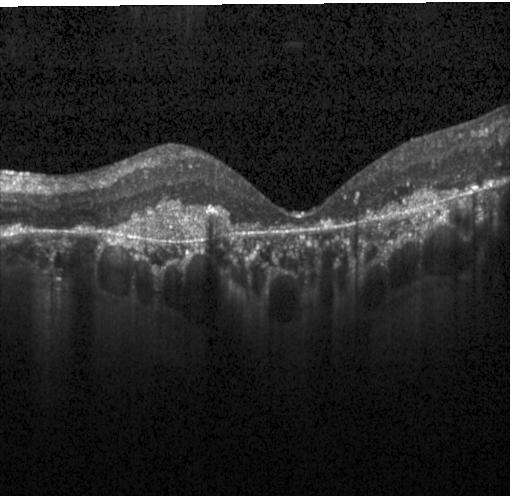 Finding: a choroidal neovascular membrane.